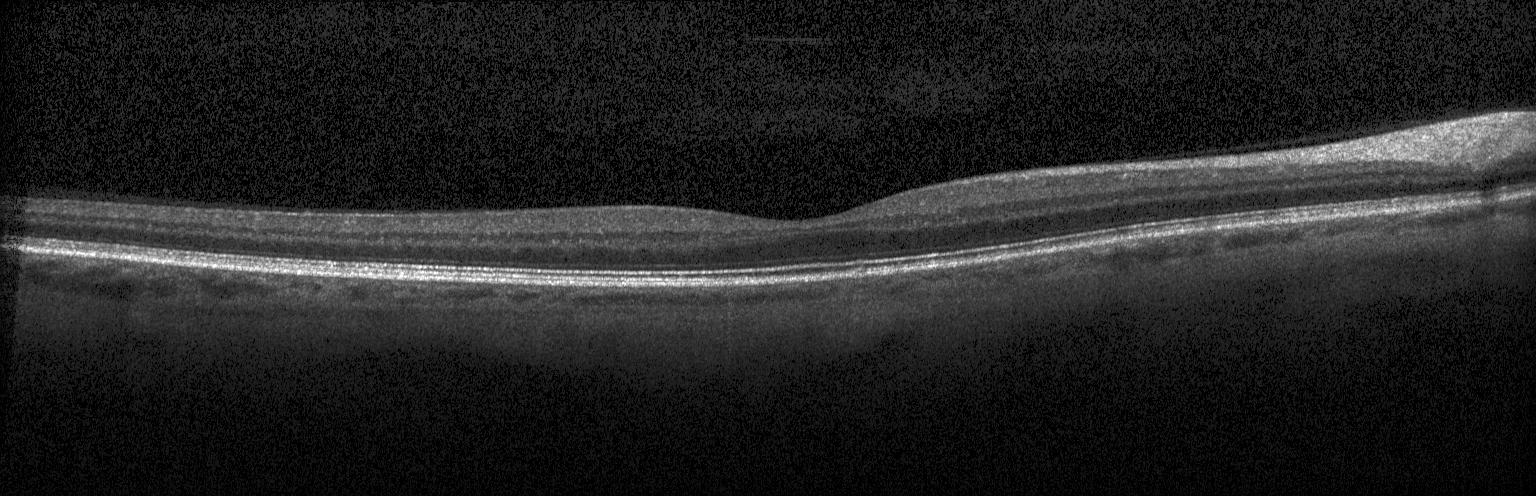
Impression: no evidence of choroidal neovascularization, diabetic macular edema, or drusen.